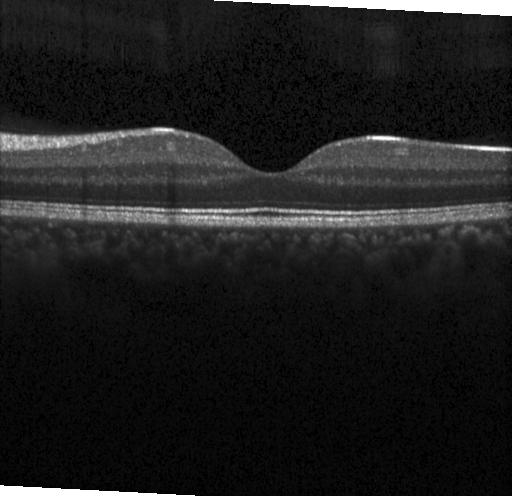

Fovea-centered, OCT B-scan, Heidelberg Spectralis. Diagnosis: no CNV, no DME, and no drusen.